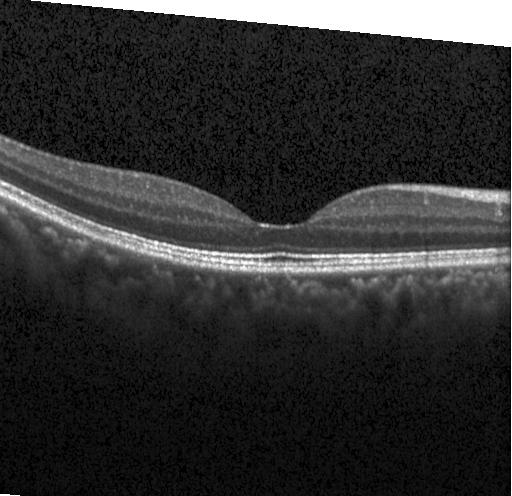

Centered on the fovea · Heidelberg Spectralis · optical coherence tomography scan
Diagnosis: no choroidal neovascularization, no diabetic macular edema, and no drusen.